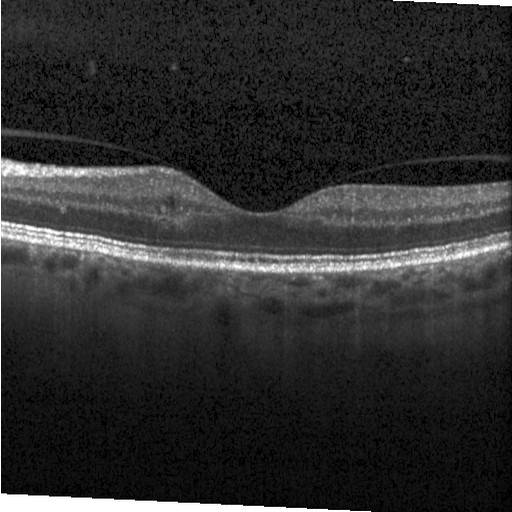 Impression: diabetic macular edema (DME).